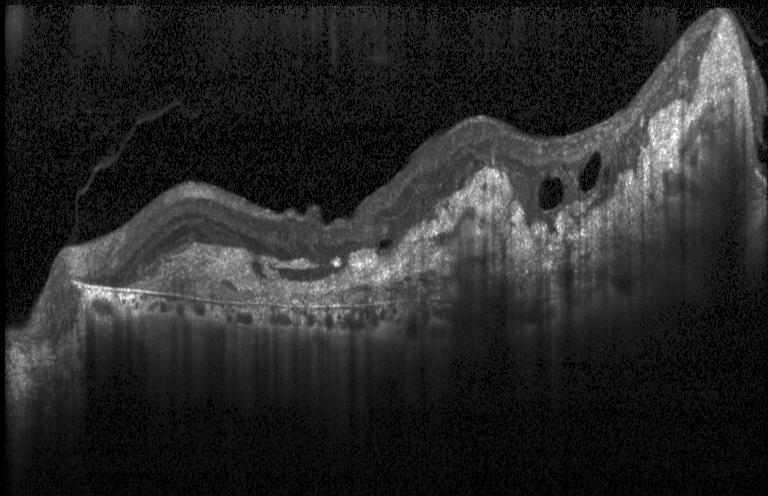
Finding: a choroidal neovascular membrane.